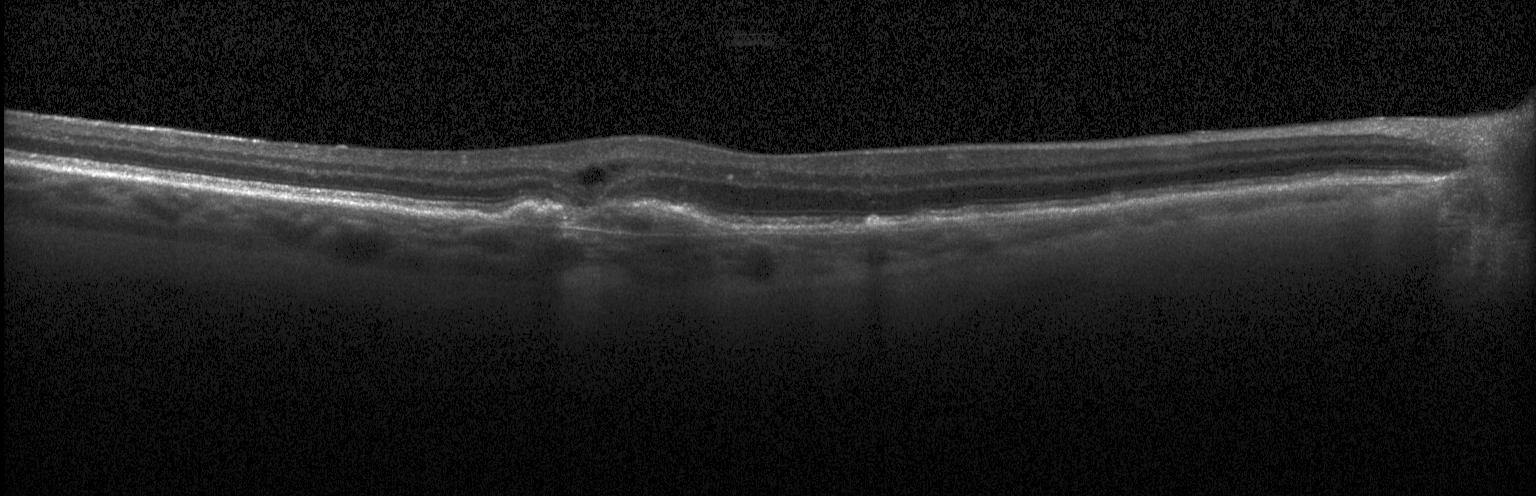

Optical coherence tomography B-scan. Acquired on a Heidelberg Spectralis.
Finding: a choroidal neovascular membrane.